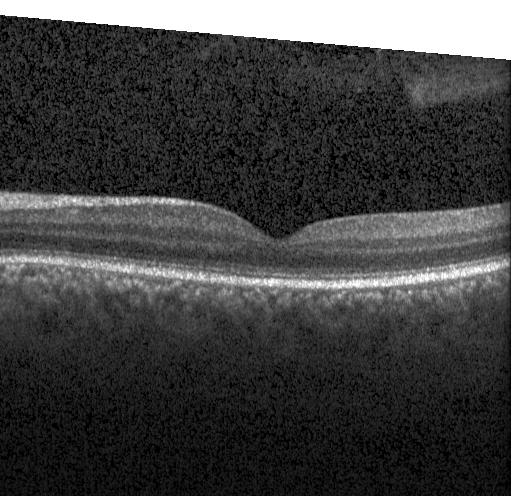

OCT B-scan · fovea-centered · SD-OCT.
Diagnosis: no CNV, DME, or drusen.